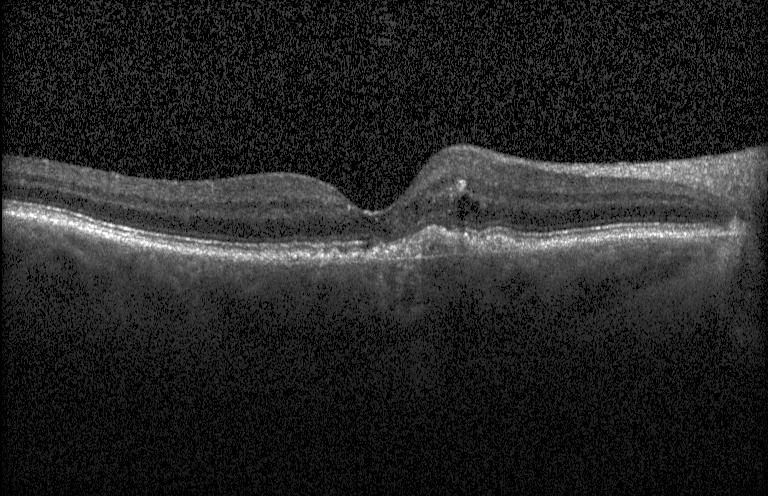
Finding: choroidal neovascularization (CNV).